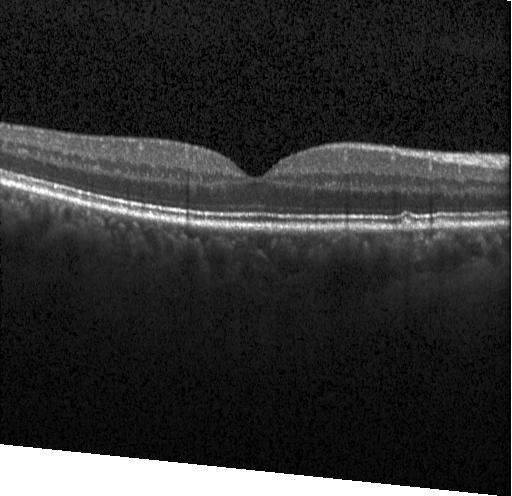
Acquired on a Heidelberg Spectralis · retinal OCT B-scan · SD-OCT · horizontal scan through the fovea
Diagnosis: drusen.